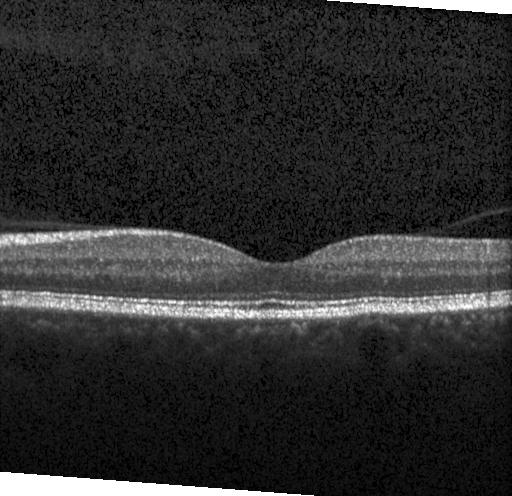

Spectral-domain OCT; OCT line scan; centered on the fovea; Heidelberg Spectralis OCT system
Finding: no CNV, DME, or drusen.